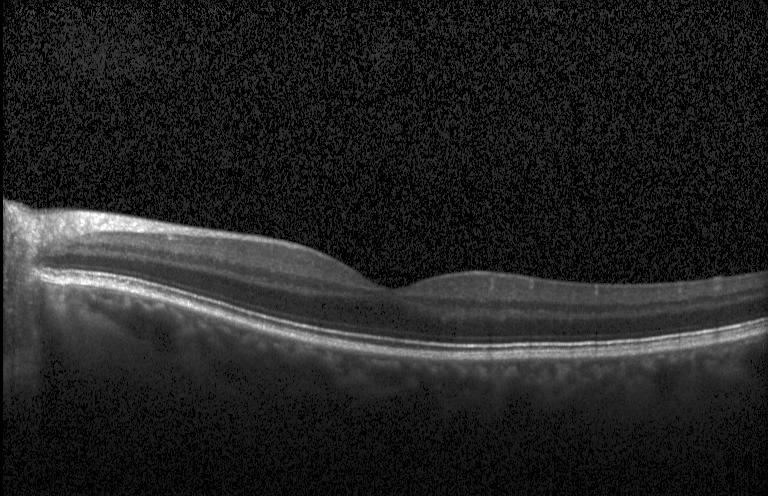
Retinal OCT B-scan.
Impression: neither choroidal neovascularization, diabetic macular edema, nor drusen.